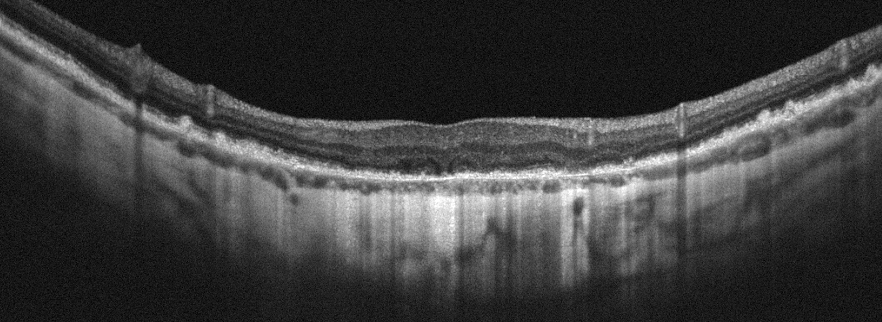

OCT finding: age-related macular degeneration.